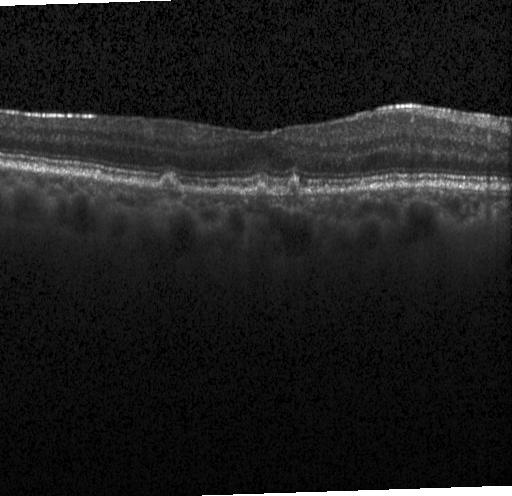
Centered on the fovea, spectral-domain optical coherence tomography, OCT line scan, acquired on a Heidelberg Spectralis — Assessment: drusen.